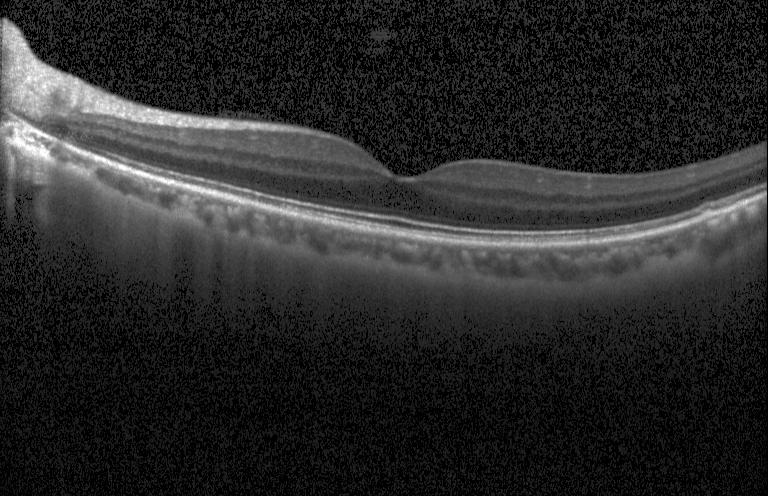
OCT scan showing neither choroidal neovascularization, diabetic macular edema, nor drusen.